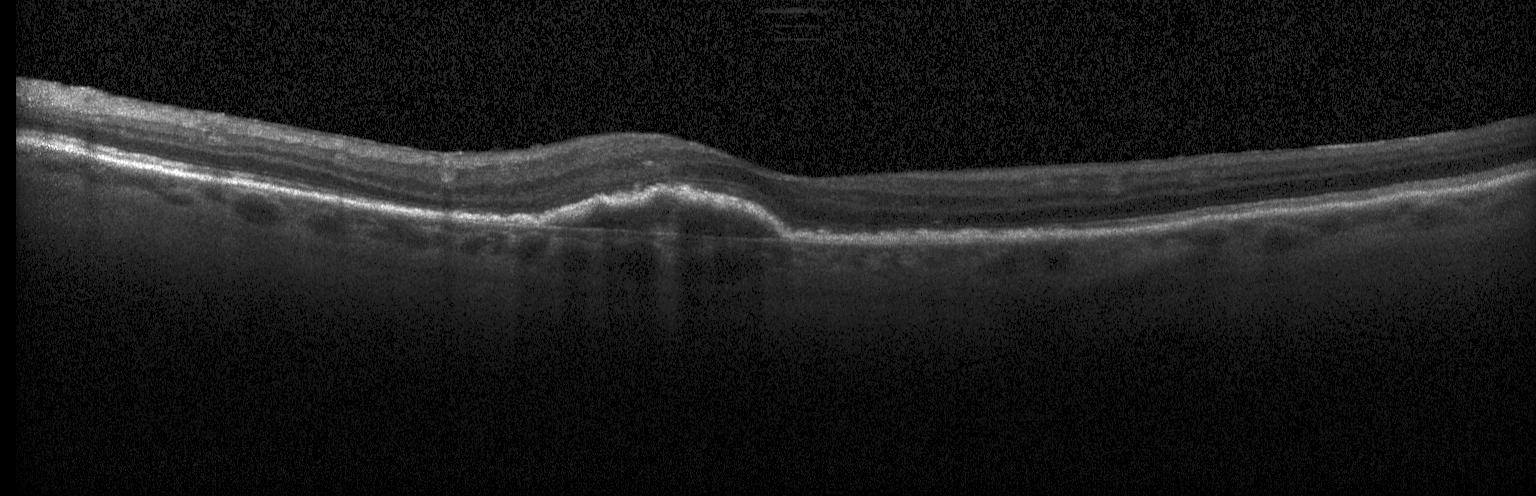 Dx: CNV.